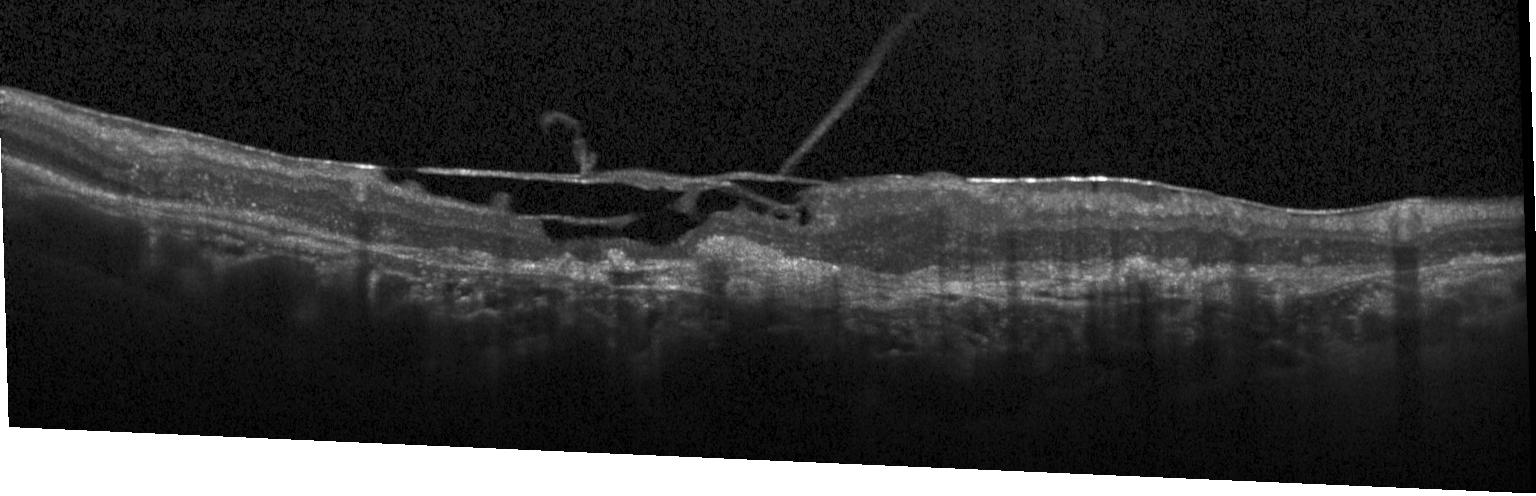 Spectral-domain optical coherence tomography · optical coherence tomography B-scan — Diagnosis: a choroidal neovascular membrane.